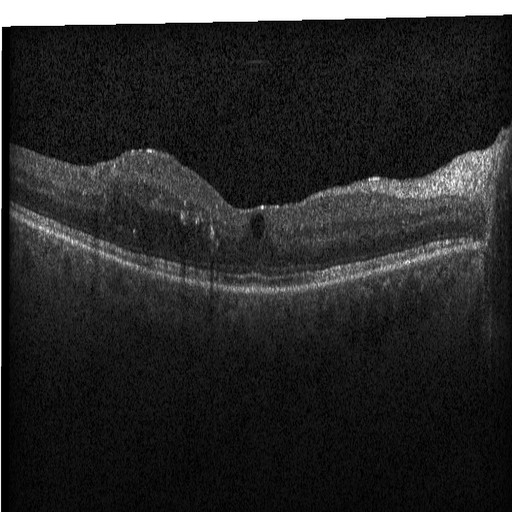 Acquired on a Heidelberg Spectralis · retinal OCT B-scan
Impression: diabetic macular edema (DME).